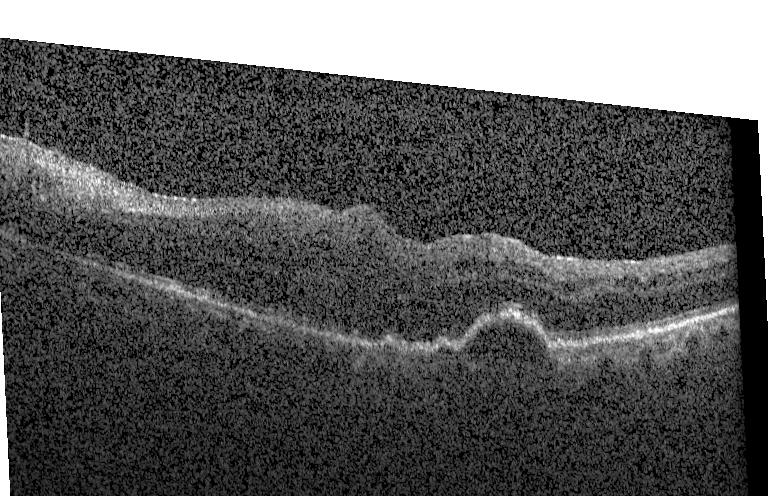

Retinal OCT B-scan, Heidelberg Spectralis, spectral-domain OCT, horizontal scan through the fovea
Macular OCT: choroidal neovascularization.